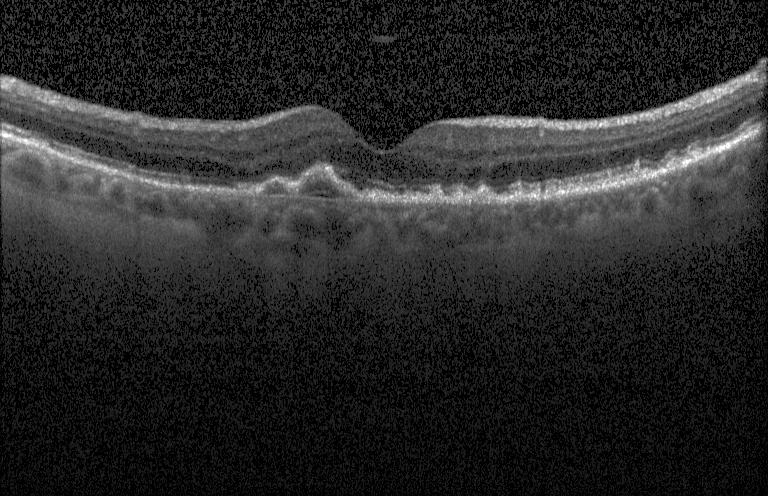

Macular OCT: a choroidal neovascular membrane.